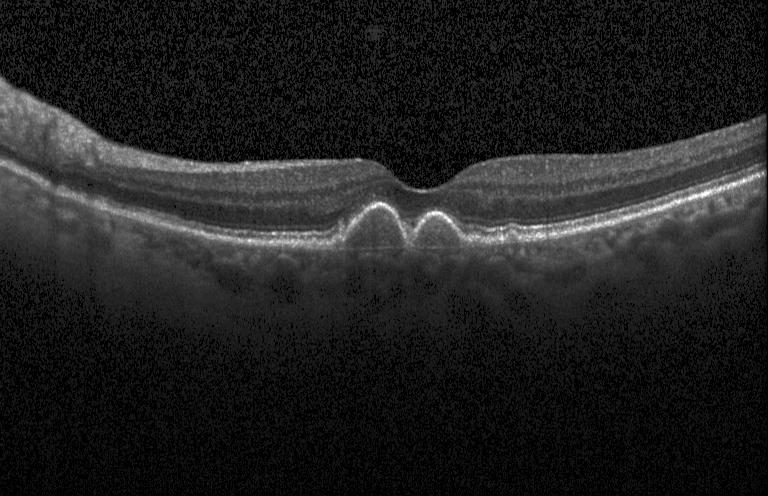

Macular OCT demonstrating multiple drusen.